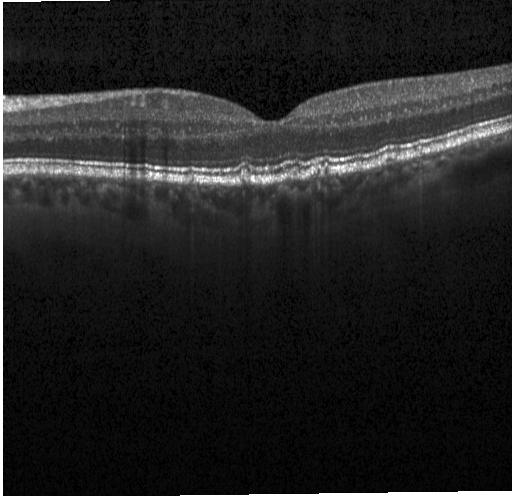 SD-OCT; optical coherence tomography scan
Finding: multiple drusen.